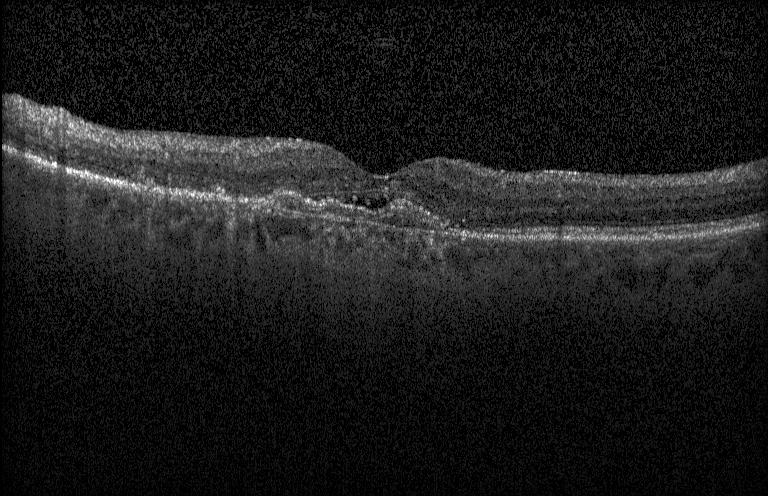 Finding: a choroidal neovascular membrane.